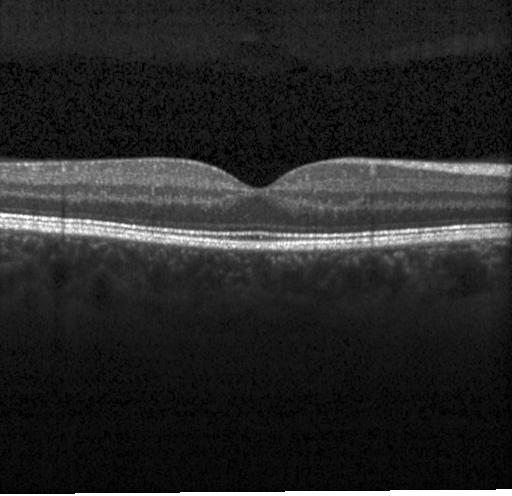

Heidelberg Spectralis · horizontal scan through the fovea · spectral-domain OCT · OCT B-scan — Finding: no evidence of choroidal neovascularization, diabetic macular edema, or drusen.